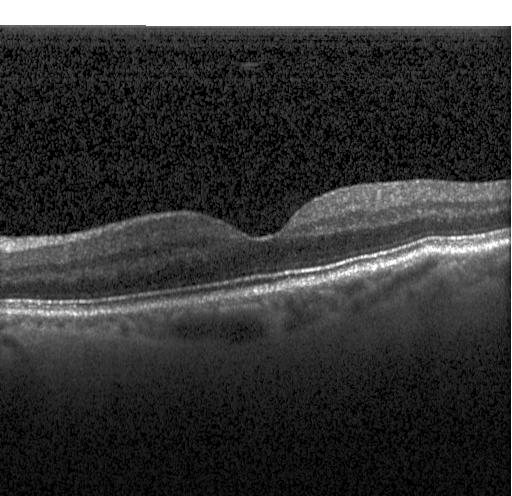

Spectral-domain OCT. Heidelberg Spectralis OCT system. Retinal OCT B-scan. Assessment: neither CNV, DME, nor drusen.